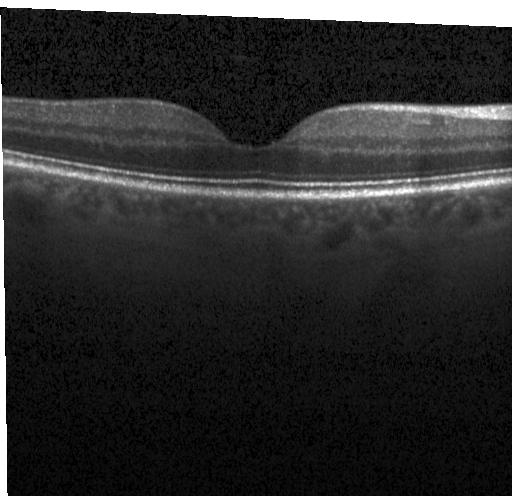
Impression: no choroidal neovascularization, no diabetic macular edema, and no drusen.